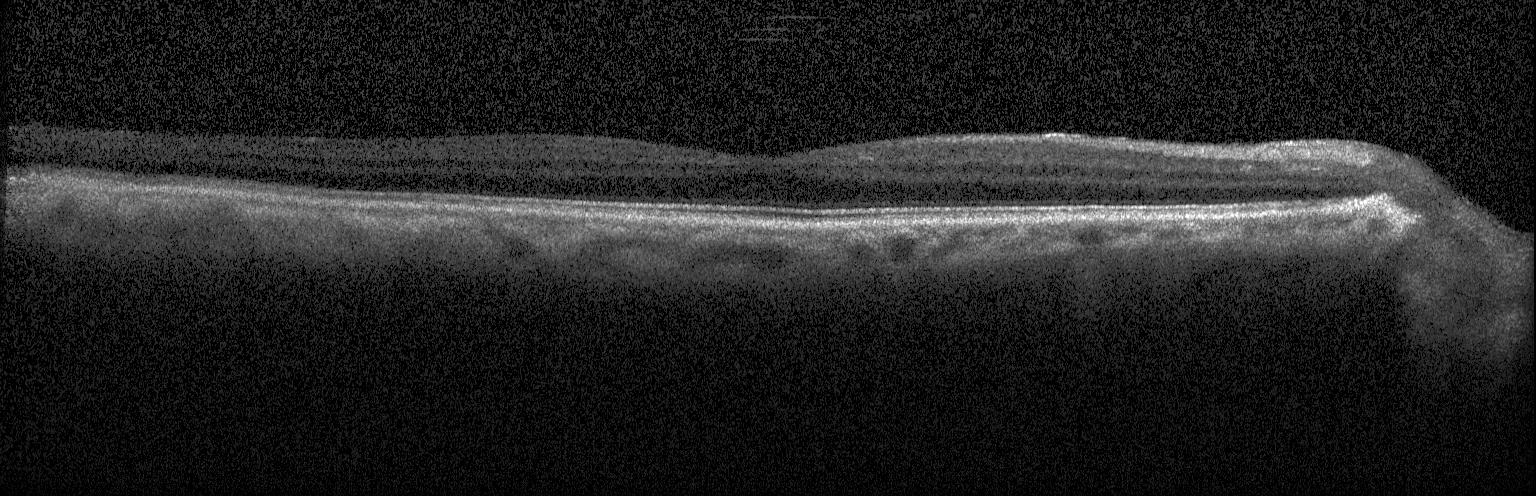
SD-OCT, optical coherence tomography scan. The scan shows no choroidal neovascularization, no diabetic macular edema, and no drusen.